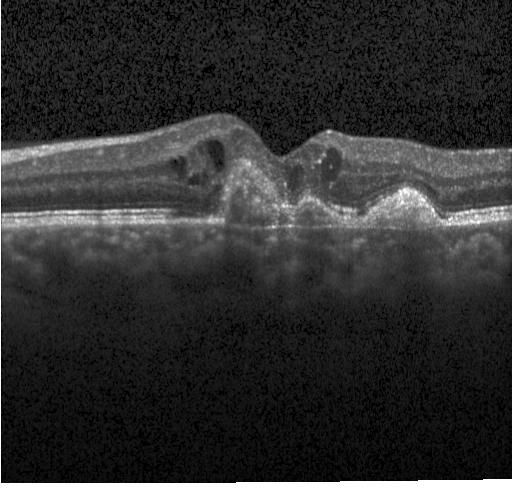 Macular scan · retinal OCT B-scan.
Macular OCT: a choroidal neovascular membrane.